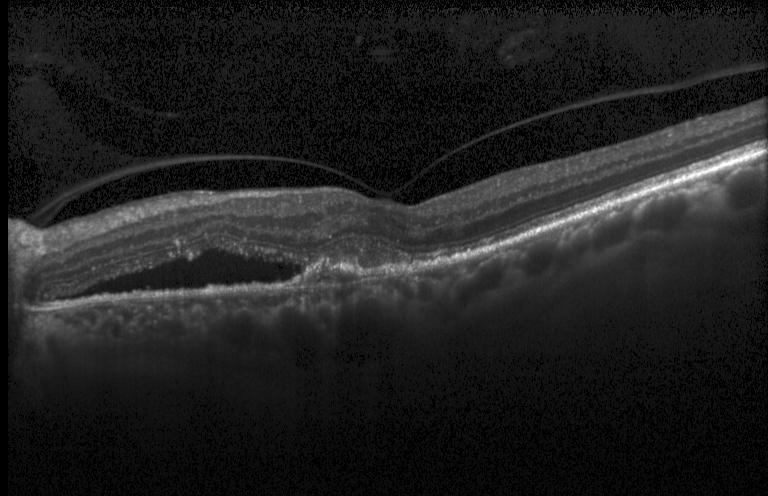
Optical coherence tomography scan.
OCT finding: a choroidal neovascular membrane.